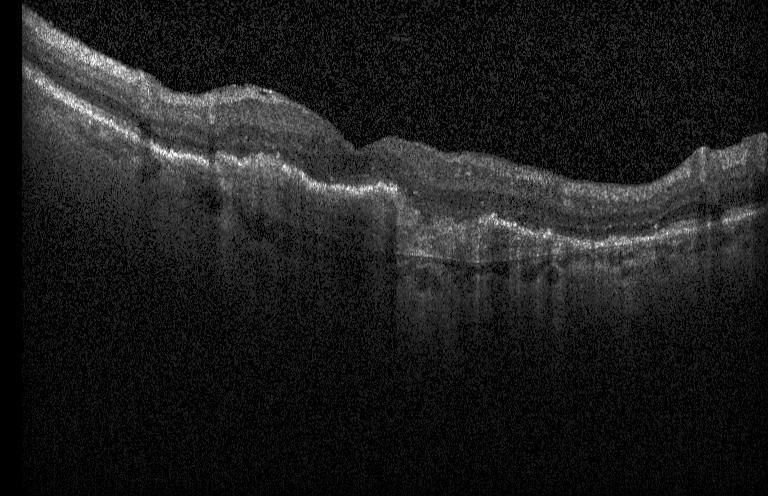

SD-OCT · OCT B-scan · Heidelberg Spectralis · horizontal scan through the fovea
Impression: a choroidal neovascular membrane.